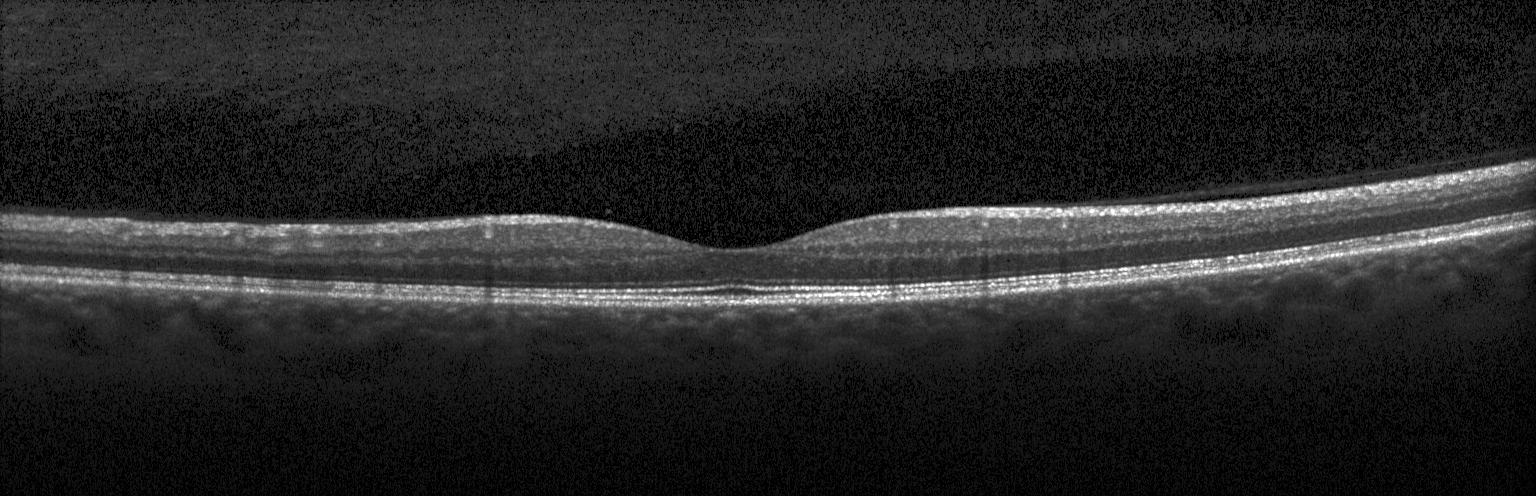
Instrument: Heidelberg Spectralis; OCT B-scan; spectral-domain OCT — This B-scan demonstrates no choroidal neovascularization, no diabetic macular edema, and no drusen.